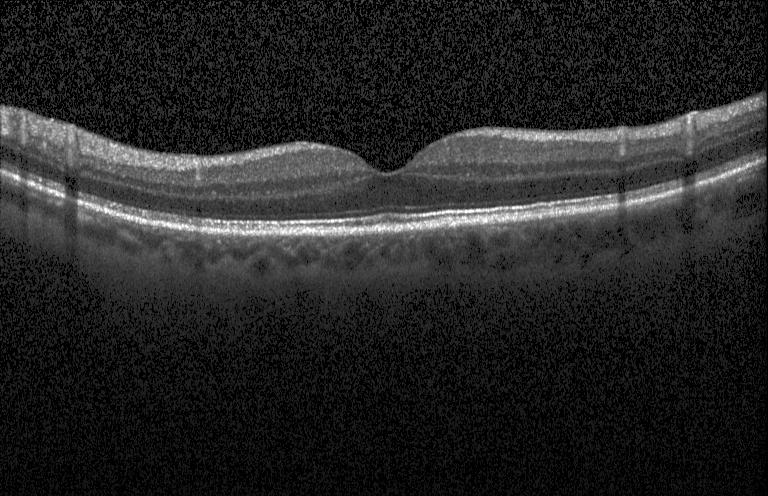 Spectral-domain OCT, optical coherence tomography B-scan, through the macula, instrument: Heidelberg Spectralis
Diagnosis: no choroidal neovascularization, no diabetic macular edema, and no drusen.